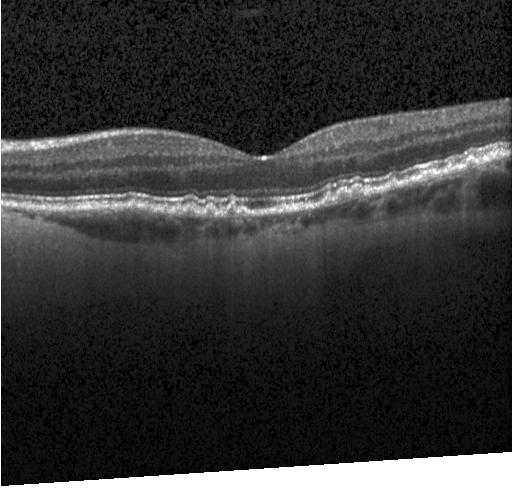 SD-OCT, retinal OCT B-scan.
Macular OCT: sub-RPE drusenoid deposits.